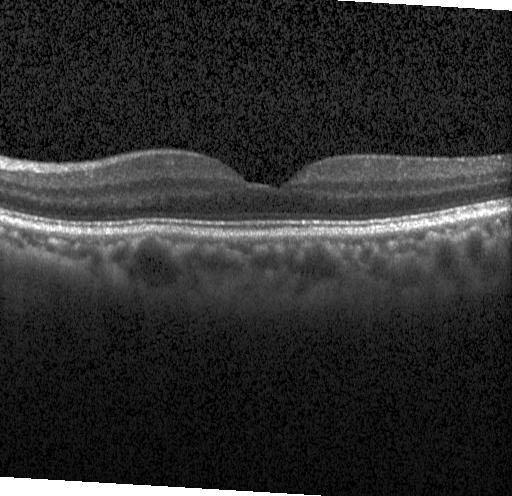 Diagnosis: no evidence of CNV, DME, or drusen.